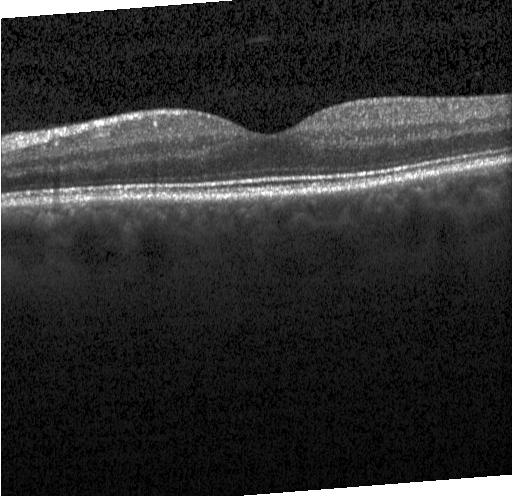

OCT line scan, horizontal scan through the fovea. Impression: no choroidal neovascularization, diabetic macular edema, or drusen.